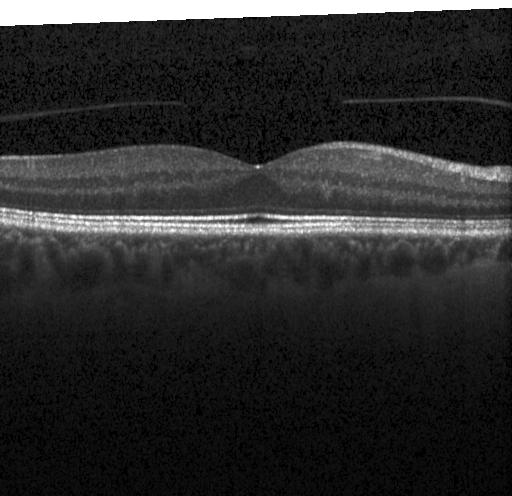 Finding: no choroidal neovascularization, no diabetic macular edema, and no drusen.